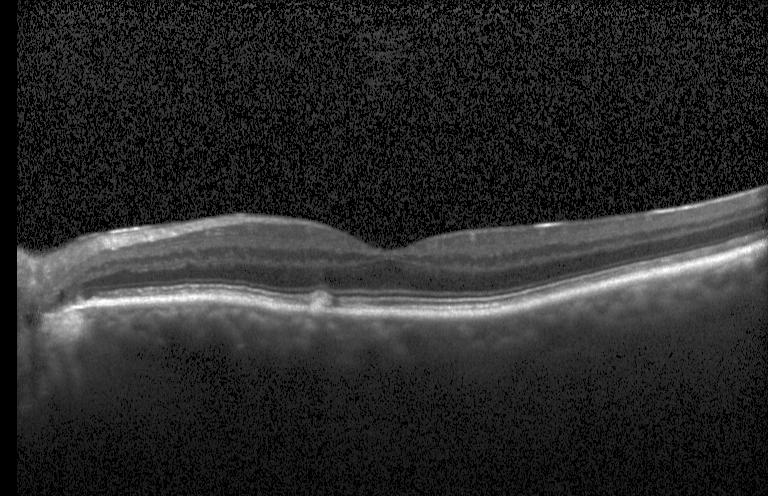
OCT line scan · Heidelberg Spectralis · spectral-domain optical coherence tomography · fovea-centered. The scan shows multiple drusen.